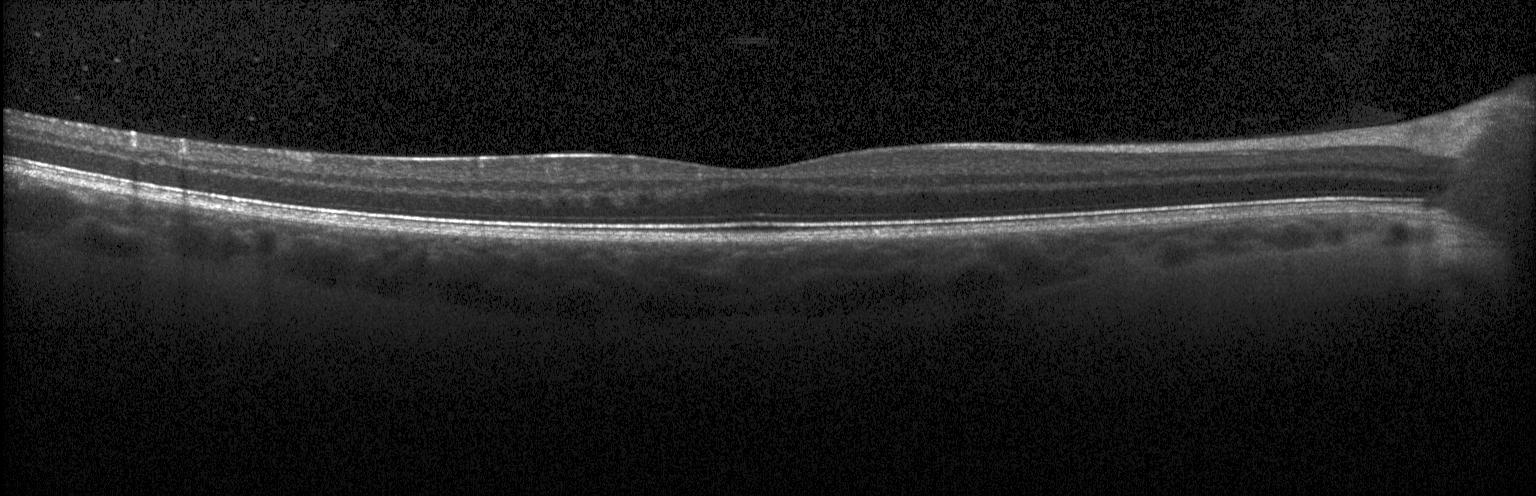
OCT B-scan, macular scan, Heidelberg Spectralis, SD-OCT. Impression: no evidence of CNV, DME, or drusen.